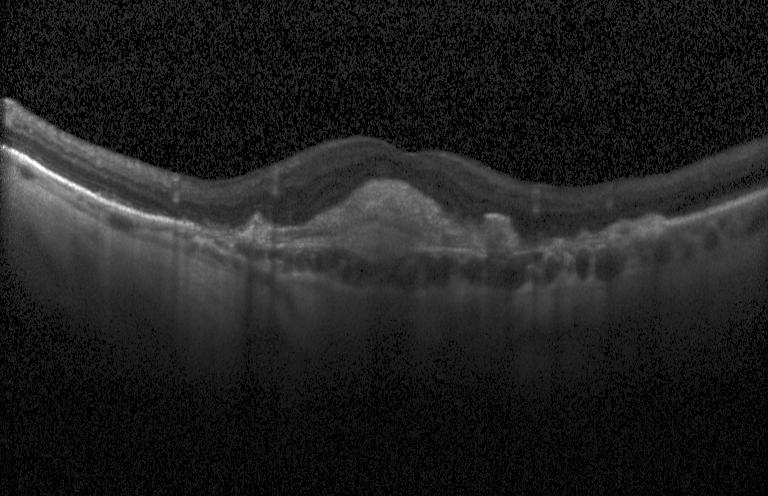 Instrument: Heidelberg Spectralis · SD-OCT · retinal OCT B-scan — Finding: choroidal neovascularization.